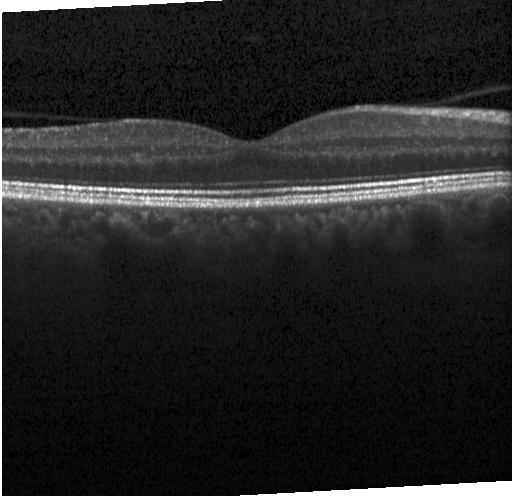

Macular OCT: no CNV, no DME, and no drusen.